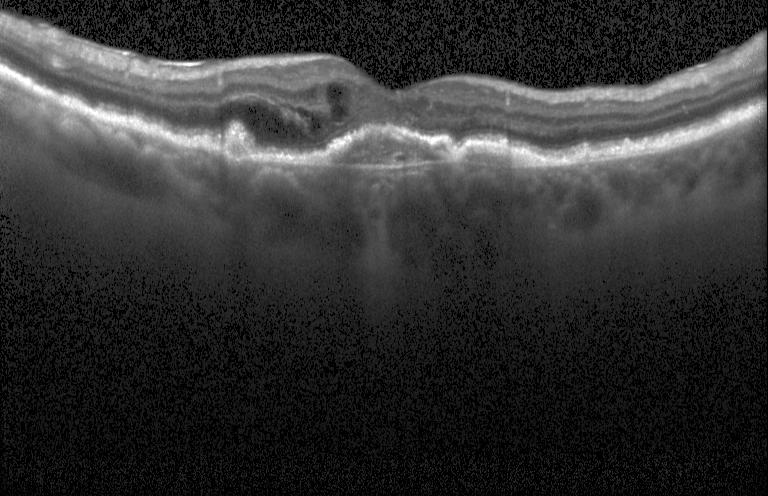

Retinal OCT B-scan
Finding: a choroidal neovascular membrane.